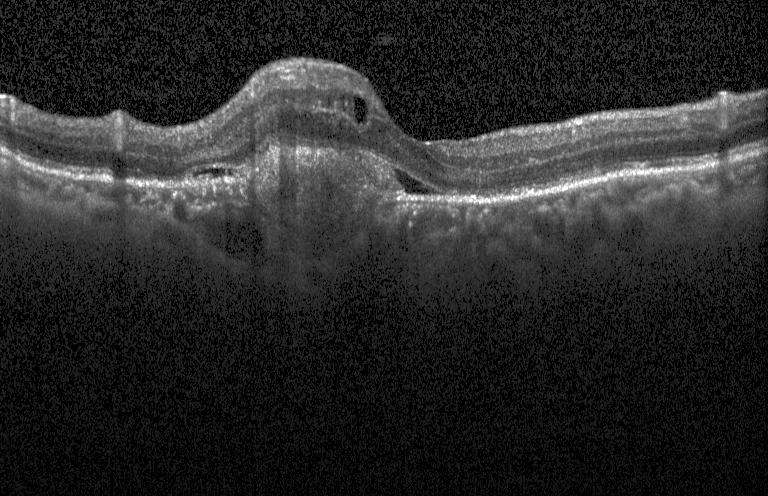
OCT B-scan — OCT finding: a choroidal neovascular membrane.